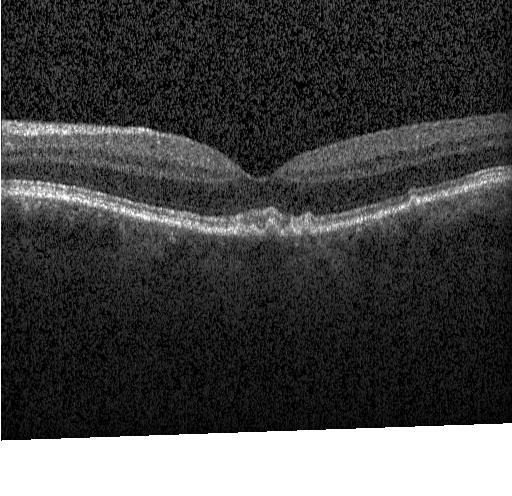
Diagnosis: multiple drusen.